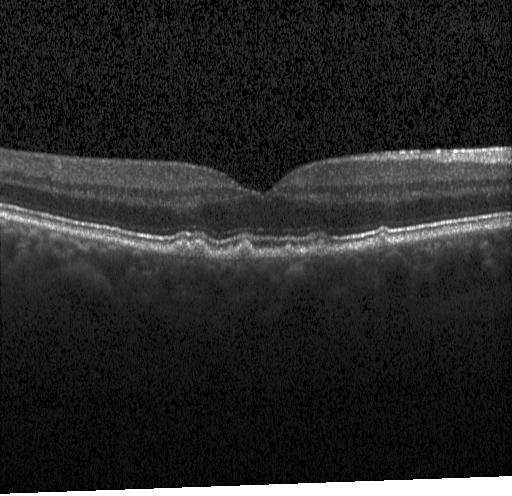
Optical coherence tomography scan. Instrument: Heidelberg Spectralis. Fovea-centered. The scan shows multiple drusen.